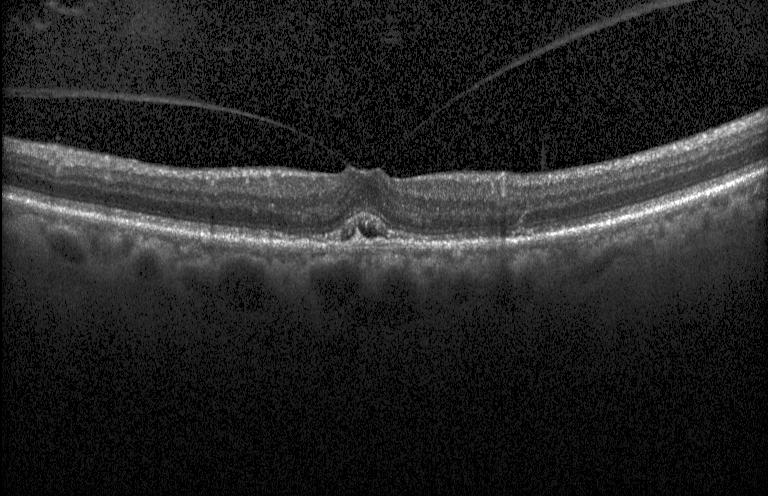 Optical coherence tomography scan, spectral-domain OCT
Diagnosis: choroidal neovascularization.